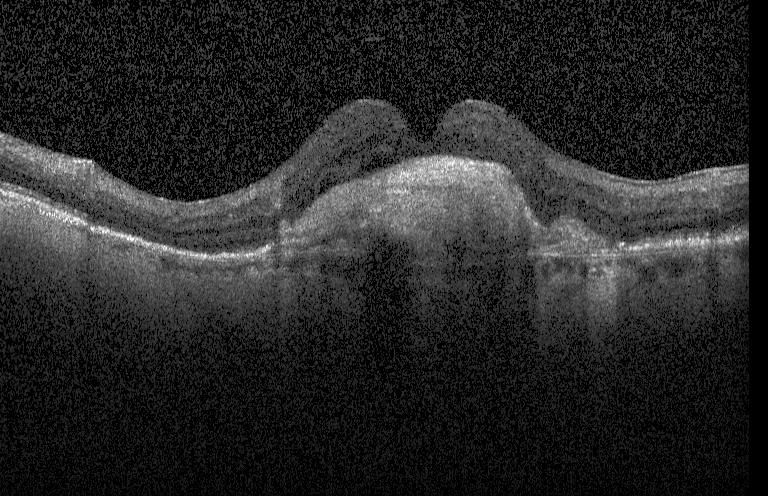

Dx: CNV.